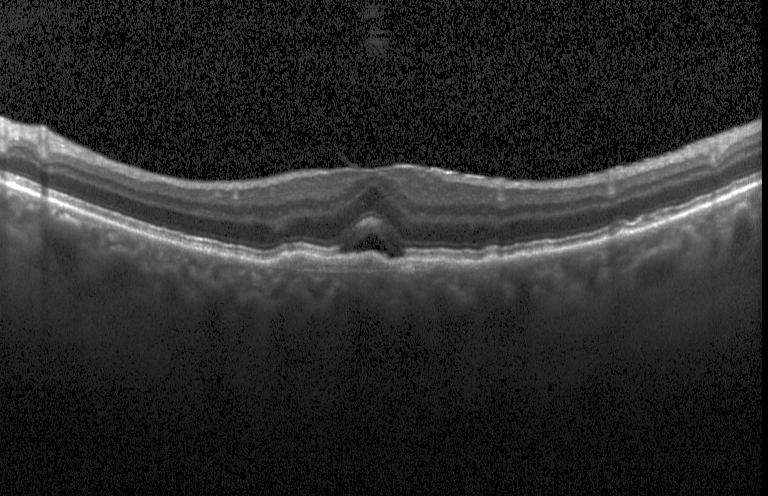

Instrument: Heidelberg Spectralis · optical coherence tomography B-scan · SD-OCT · centered on the fovea. Macular OCT: a choroidal neovascular membrane.